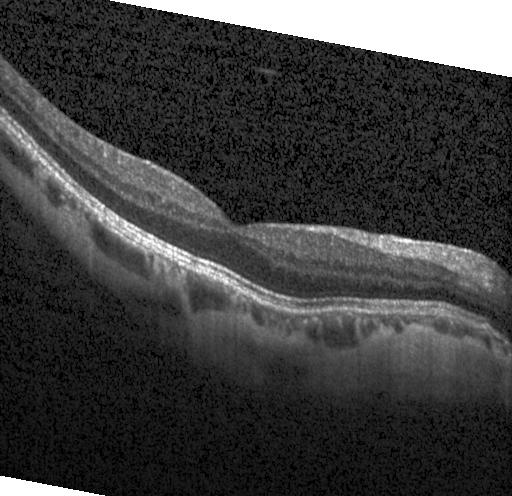 The scan shows no evidence of CNV, DME, or drusen.